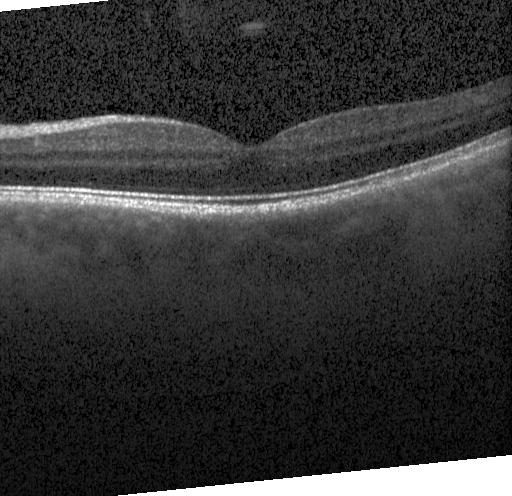
Spectral-domain optical coherence tomography, macular scan, OCT line scan, Heidelberg Spectralis OCT system.
Finding: no evidence of CNV, DME, or drusen.